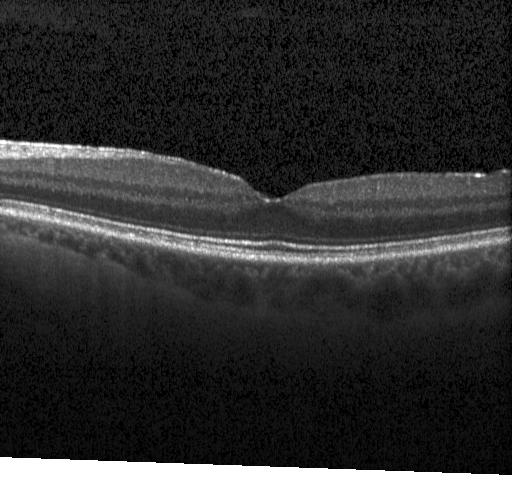

OCT B-scan. Spectral-domain OCT. Macular scan.
Diagnosis: no CNV, no DME, and no drusen.